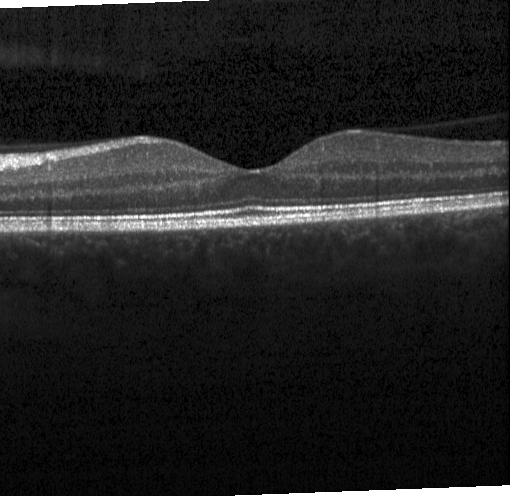 Spectral-domain OCT B-scan: neither choroidal neovascularization, diabetic macular edema, nor drusen.